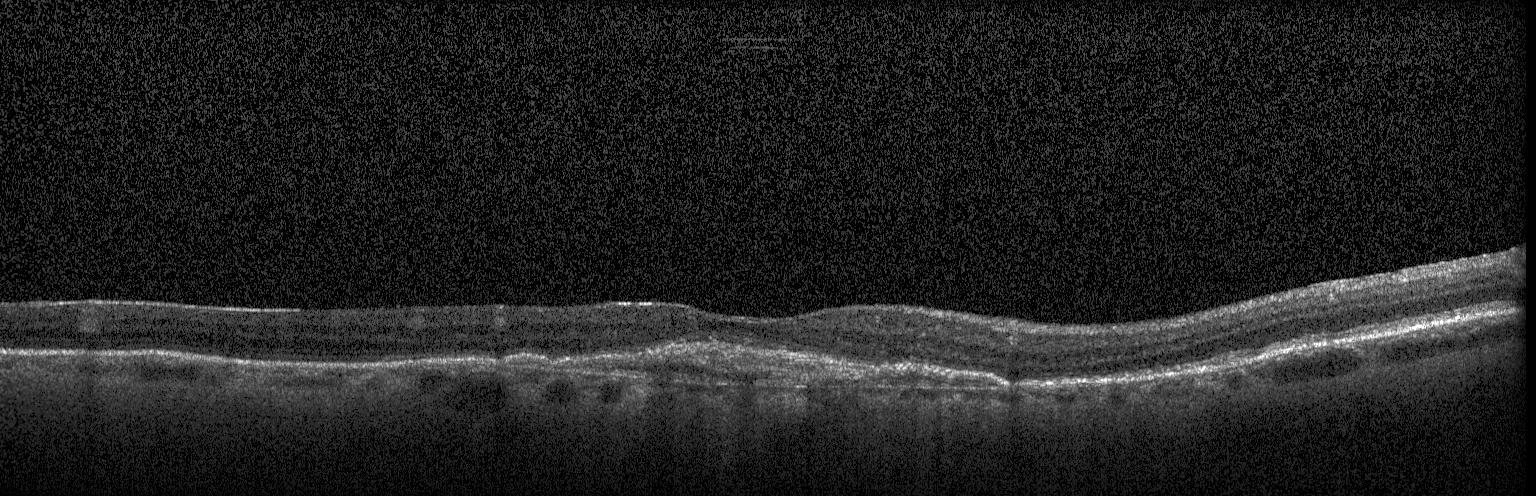 Macular OCT: choroidal neovascularization (CNV).